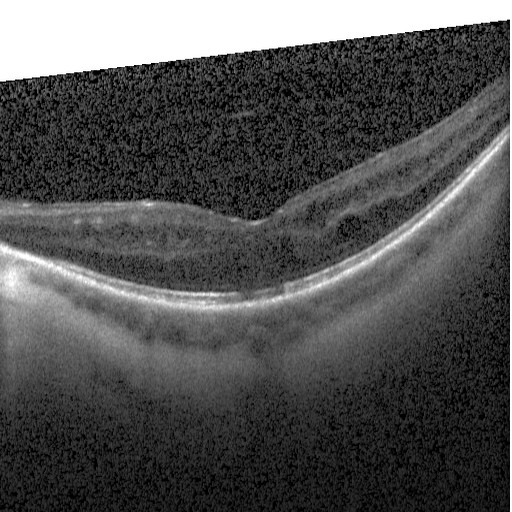
Retinal OCT cross-section. Macular OCT: diabetic macular edema.